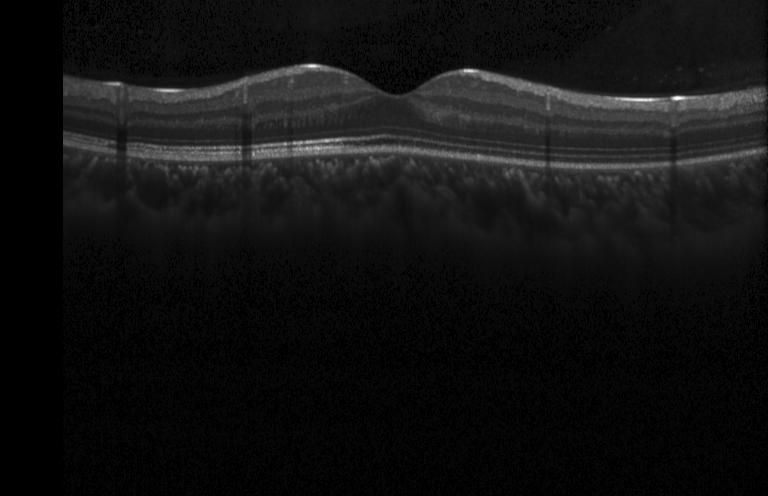

Heidelberg Spectralis OCT system; spectral-domain OCT; OCT B-scan.
Assessment: neither CNV, DME, nor drusen.